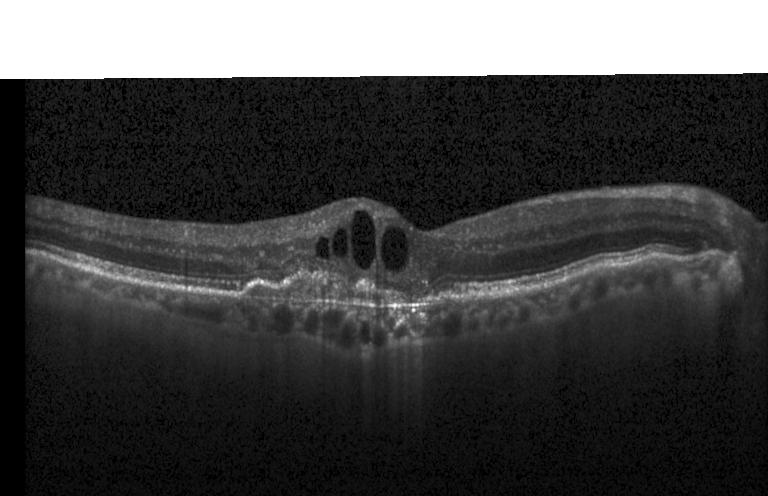 OCT finding: a choroidal neovascular membrane.